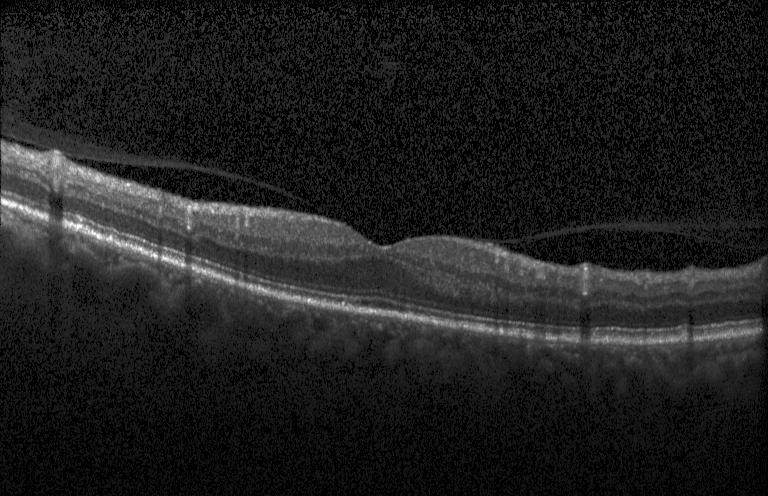

OCT B-scan · centered on the fovea — Diagnosis: no CNV, DME, or drusen.